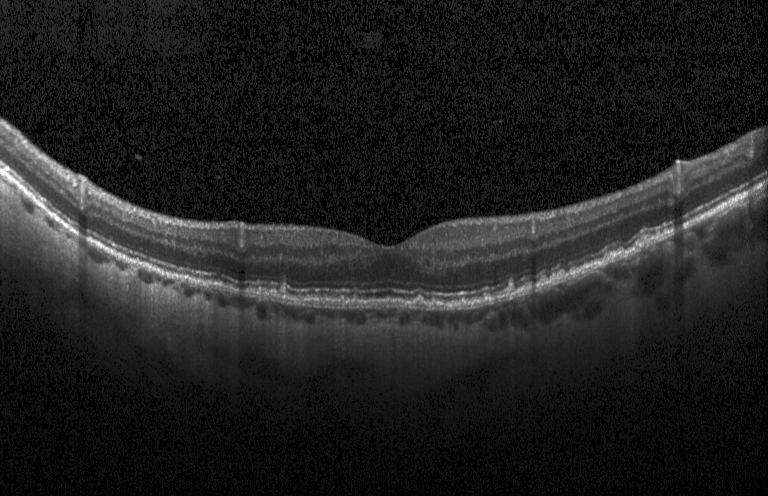 Centered on the fovea, retinal OCT B-scan
The scan shows sub-RPE drusenoid deposits.